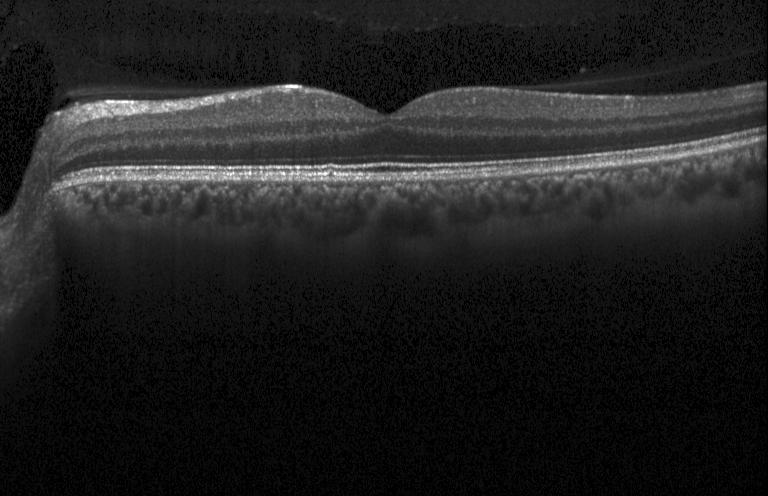
OCT B-scan — Diagnosis: no choroidal neovascularization, diabetic macular edema, or drusen.